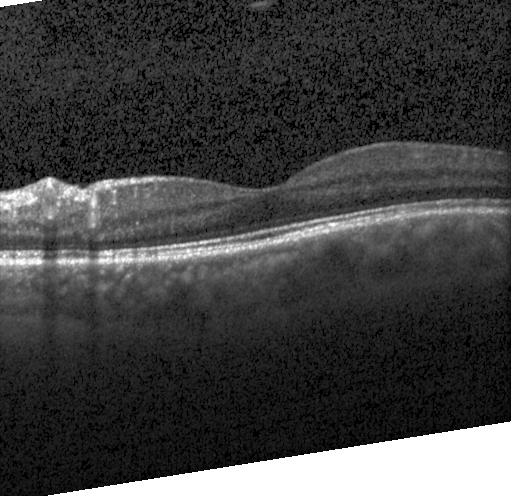 Spectral-domain optical coherence tomography, fovea-centered, Heidelberg Spectralis, retinal OCT B-scan.
Finding: no CNV, DME, or drusen.